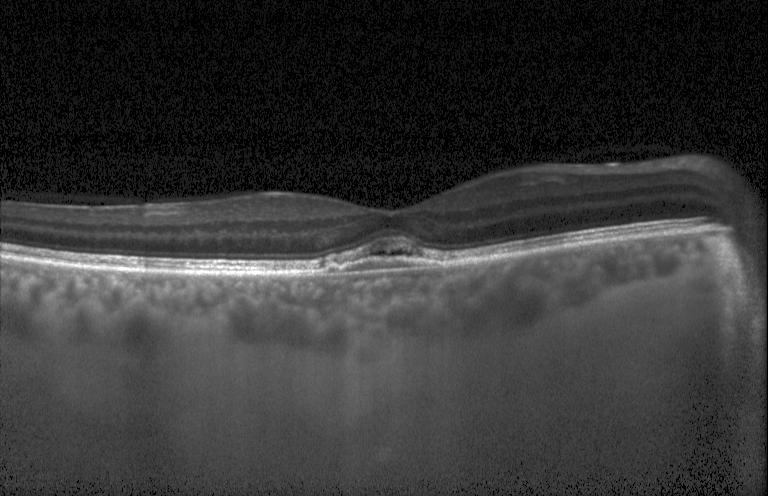 Heidelberg Spectralis; retinal OCT cross-section. Impression: a choroidal neovascular membrane.